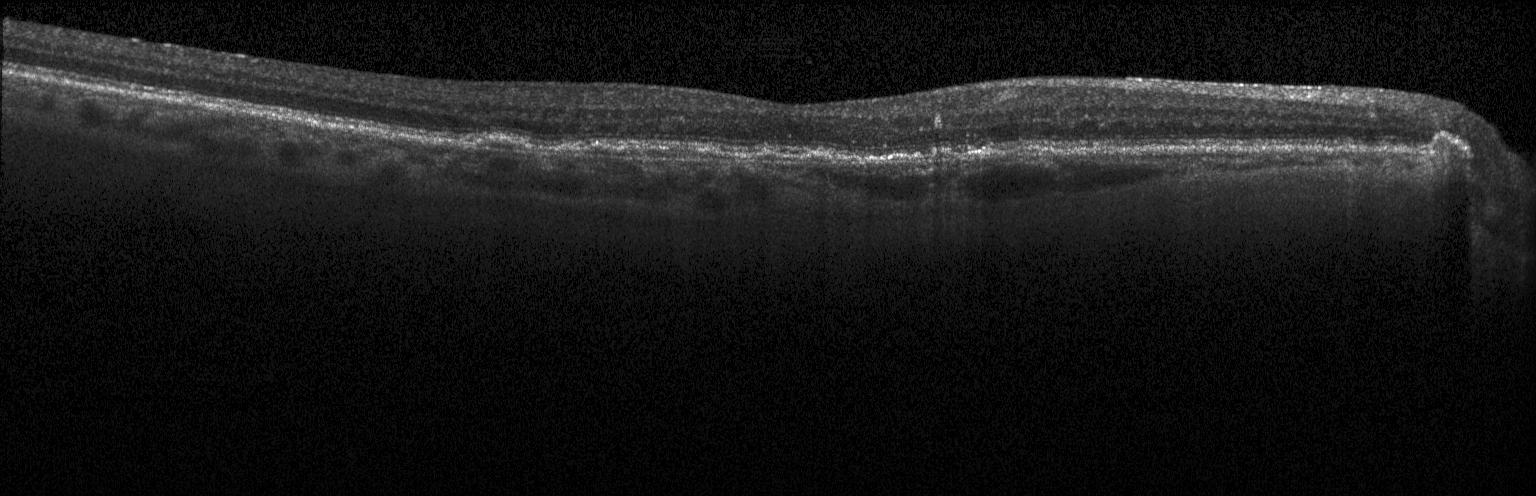

Heidelberg Spectralis OCT system; OCT B-scan; spectral-domain OCT.
Choroidal neovascularization.